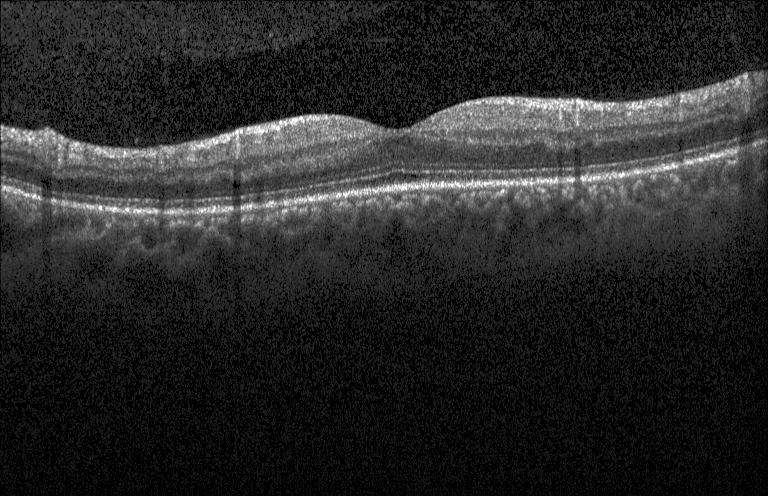 Retinal OCT B-scan. Macular scan. Instrument: Heidelberg Spectralis — Diagnosis: no choroidal neovascularization, diabetic macular edema, or drusen.